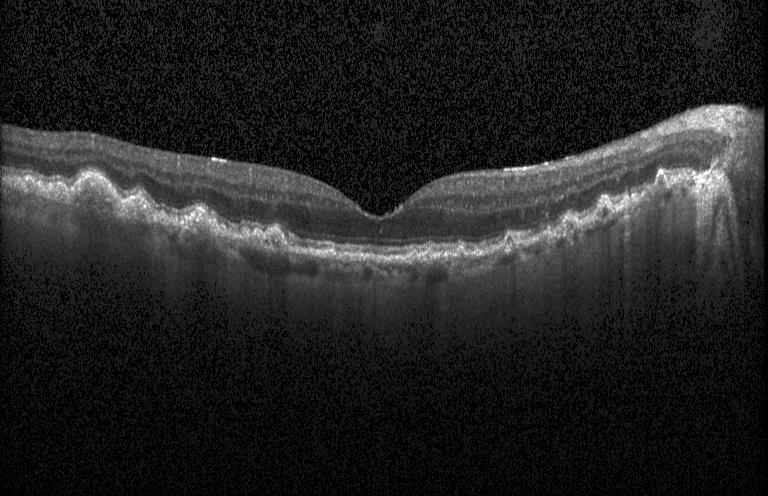
OCT B-scan.
Impression: sub-RPE drusenoid deposits.